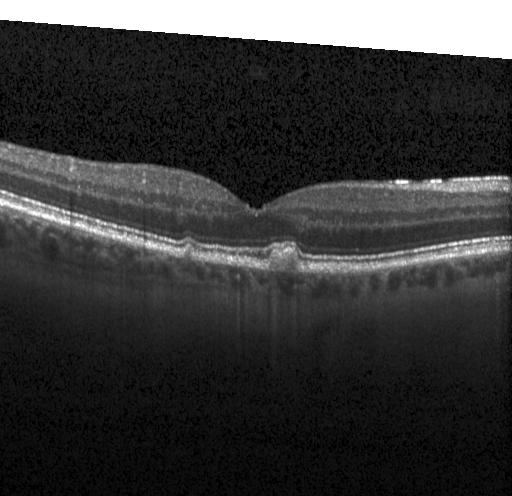 Macular OCT: multiple drusen.